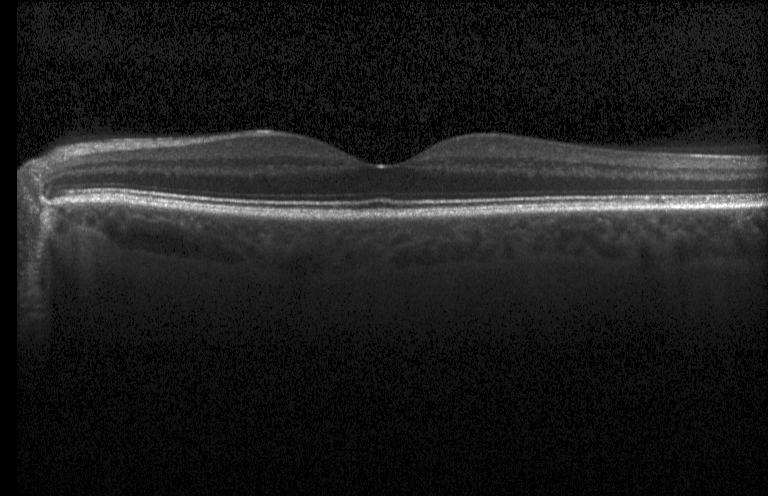

Horizontal scan through the fovea; retinal OCT cross-section; Heidelberg Spectralis.
Finding: no choroidal neovascularization, diabetic macular edema, or drusen.